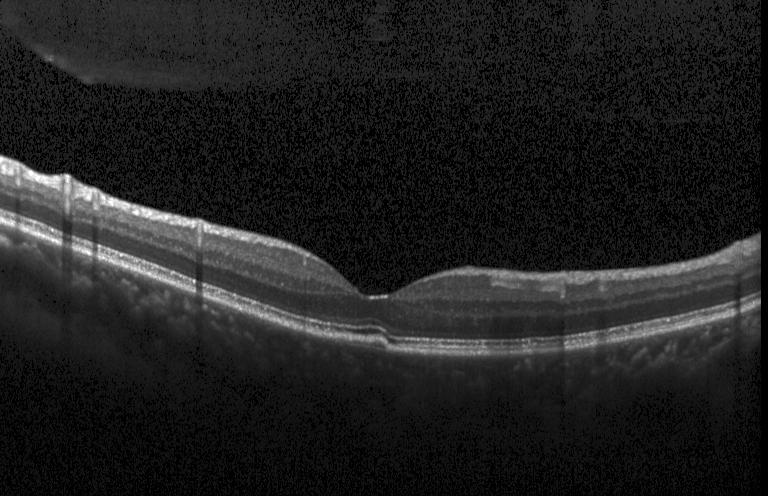 Diagnosis: drusen.